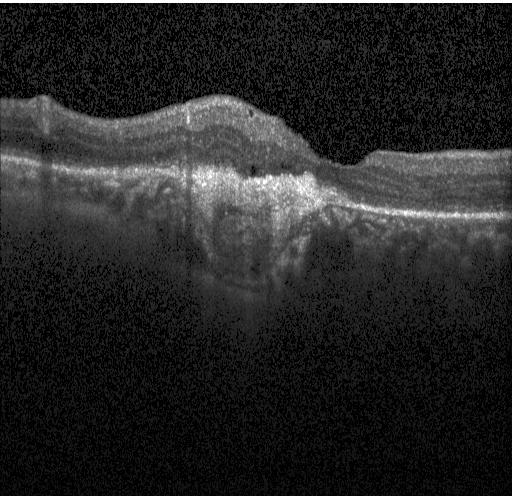 Impression: CNV.